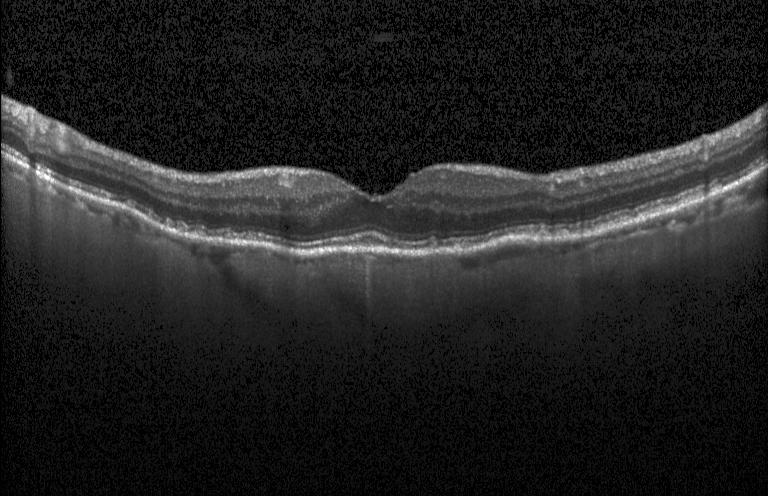

Impression: multiple drusen.